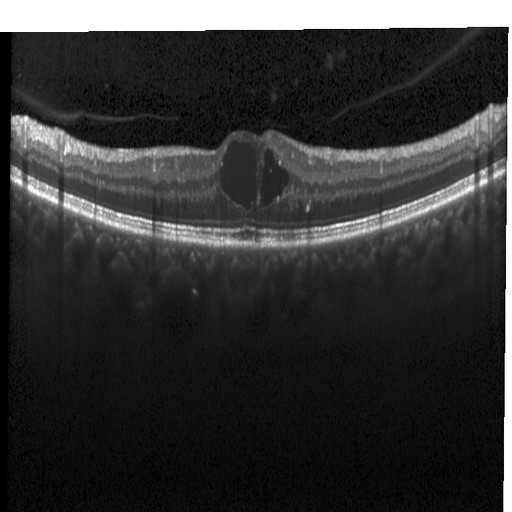 Macular OCT: diabetic macular edema (DME).